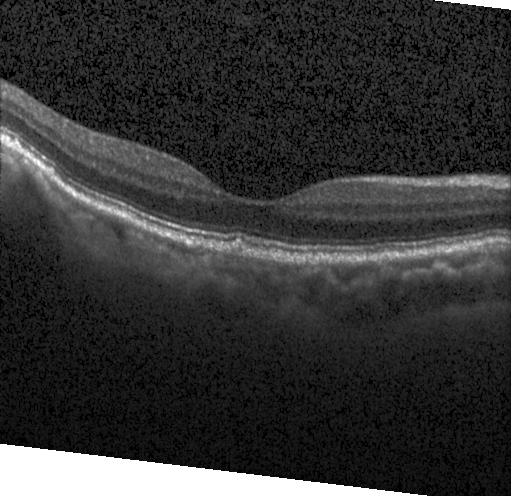

OCT B-scan.
OCT finding: no CNV, no DME, and no drusen.